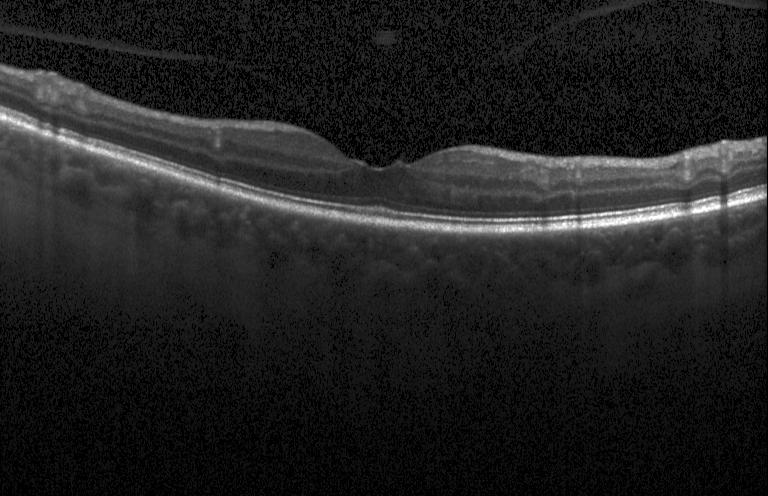
Optical coherence tomography B-scan — The scan shows no choroidal neovascularization, diabetic macular edema, or drusen.